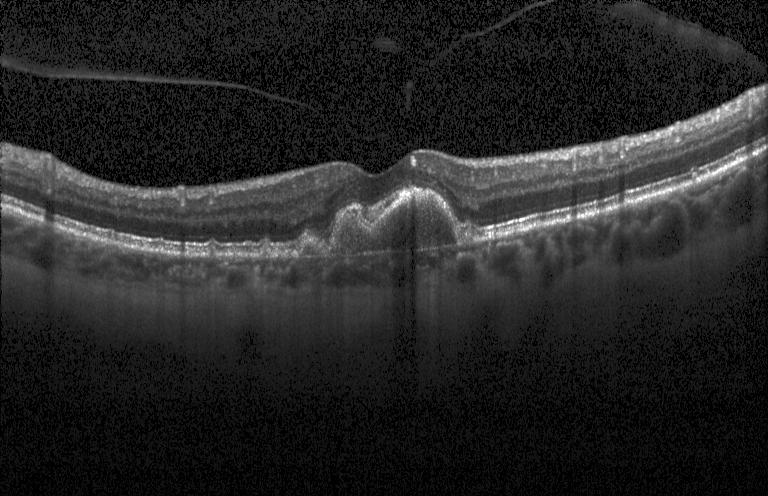 OCT B-scan; fovea-centered. Assessment: a choroidal neovascular membrane.